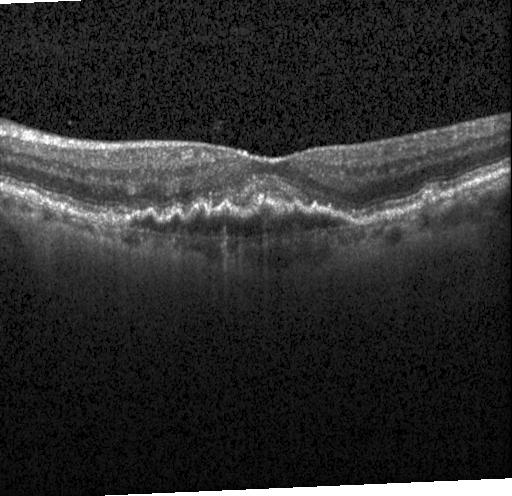

Macular scan. Optical coherence tomography scan. SD-OCT.
CNV.